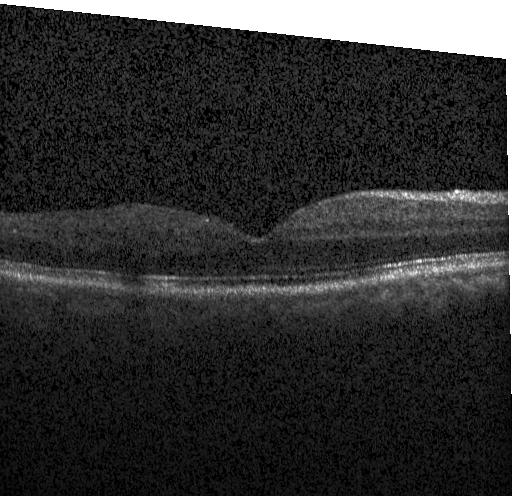
Impression: neither CNV, DME, nor drusen.